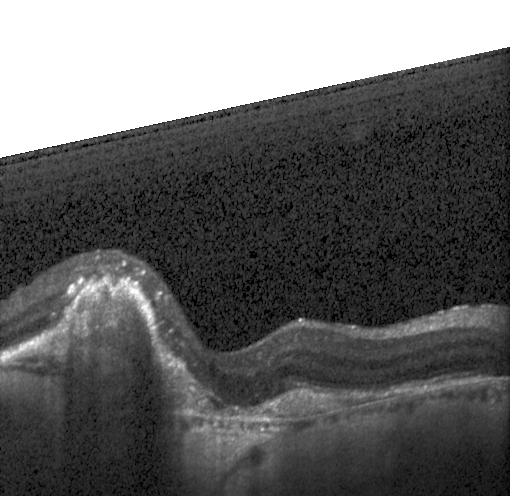
OCT scan showing a choroidal neovascular membrane.